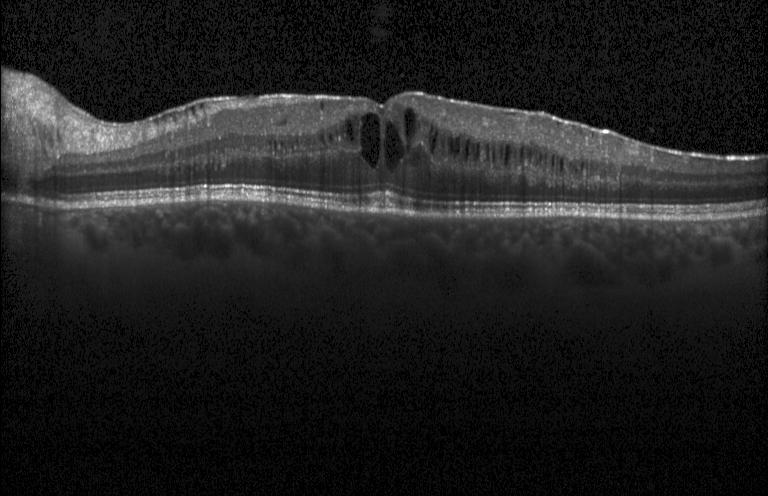
Through the macula; OCT B-scan.
DME.